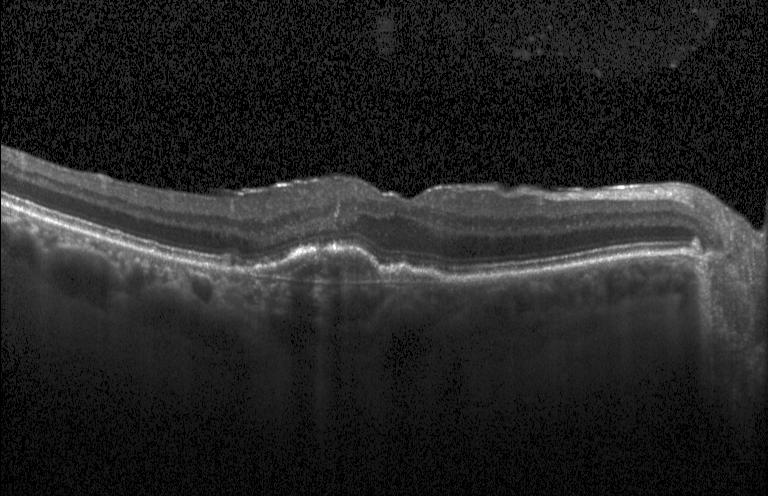 Acquired on a Heidelberg Spectralis · spectral-domain optical coherence tomography · retinal OCT cross-section · fovea-centered.
This B-scan demonstrates a choroidal neovascular membrane.